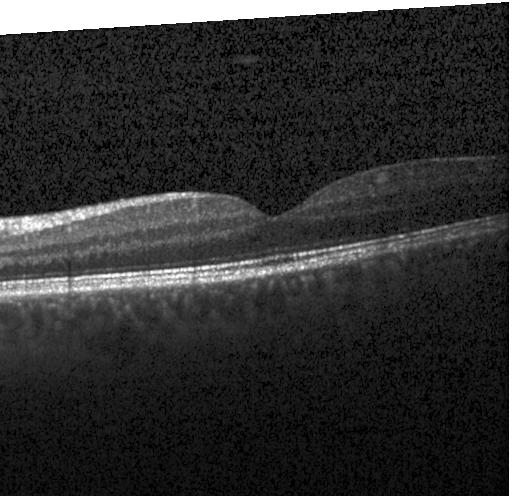 Optical coherence tomography scan. Impression: neither choroidal neovascularization, diabetic macular edema, nor drusen.